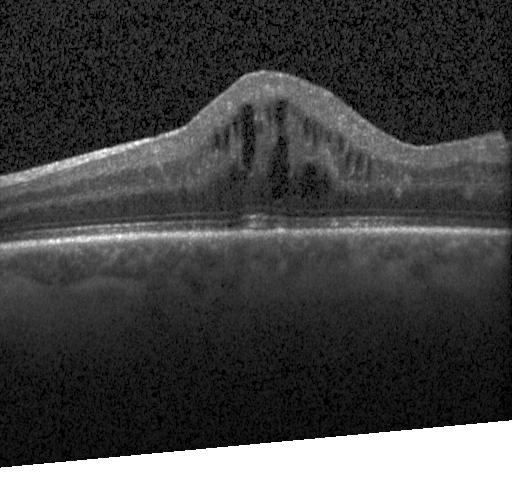

Spectral-domain OCT; retinal OCT B-scan.
Assessment: diabetic macular edema (DME).